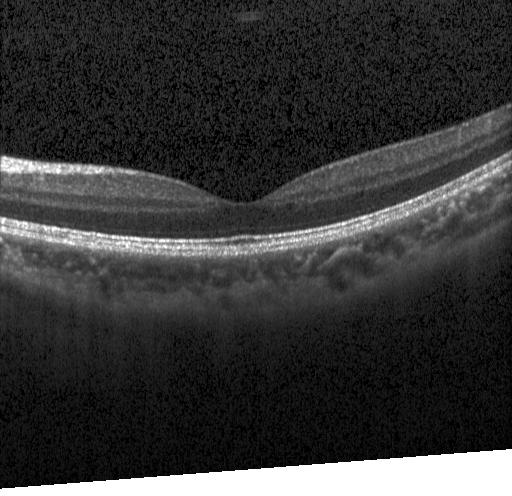

Neither choroidal neovascularization, diabetic macular edema, nor drusen.